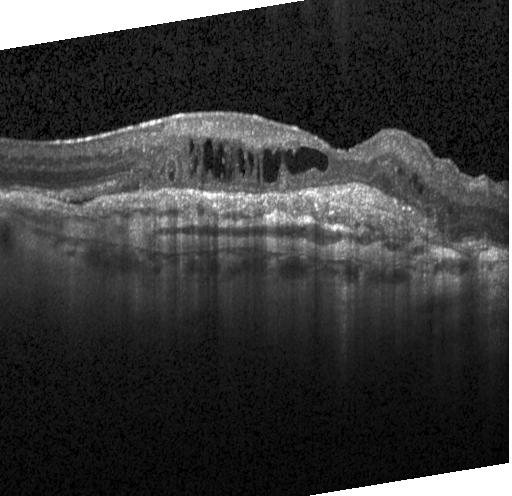
Instrument: Heidelberg Spectralis; optical coherence tomography B-scan; spectral-domain optical coherence tomography; fovea-centered — Impression: CNV.